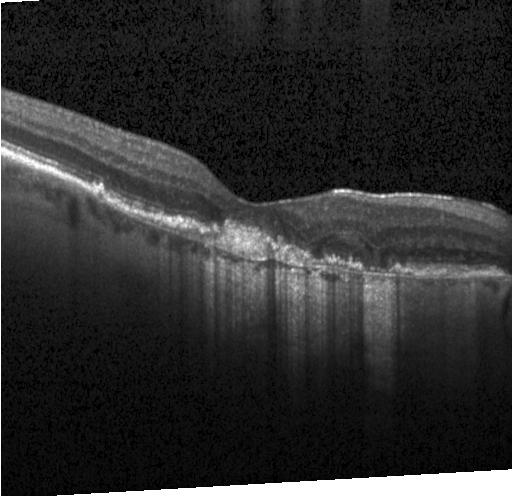 Diagnosis: CNV.